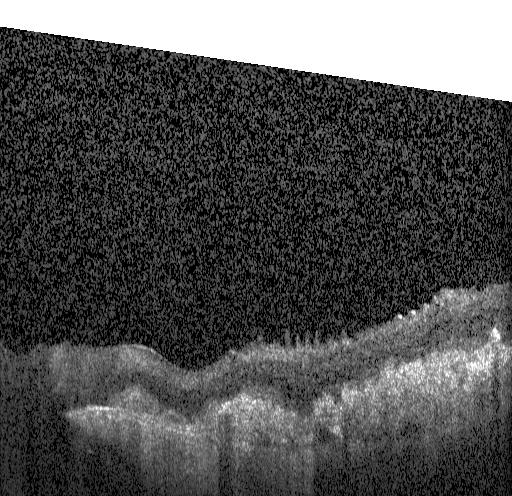

Retinal OCT cross-section showing CNV.